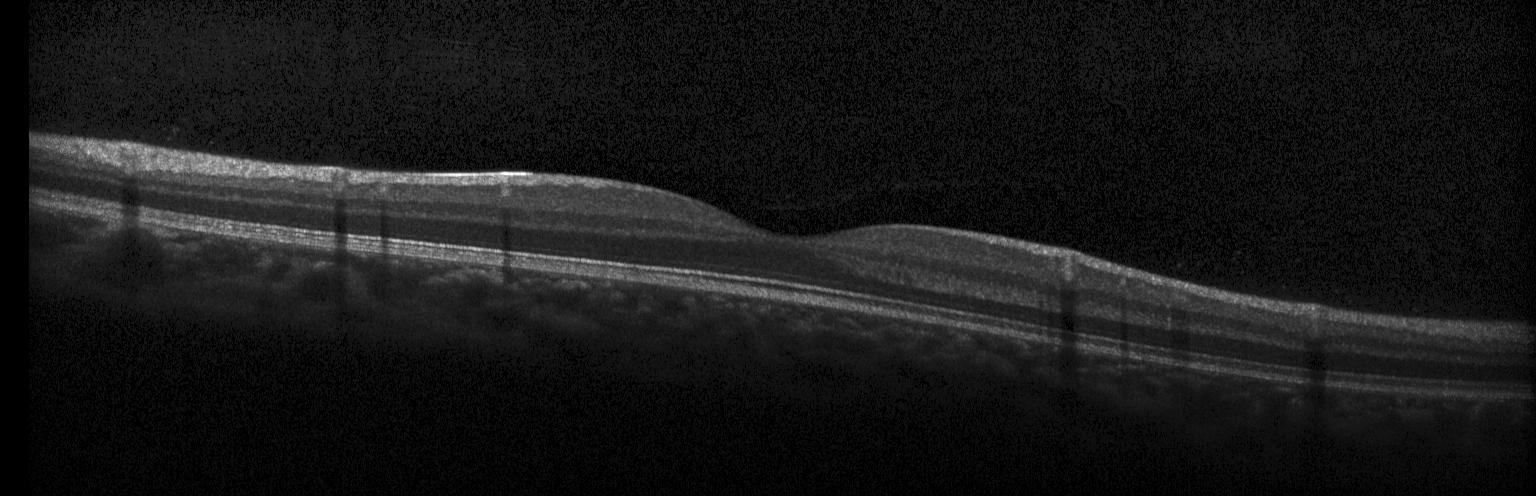

The scan shows no choroidal neovascularization, no diabetic macular edema, and no drusen.